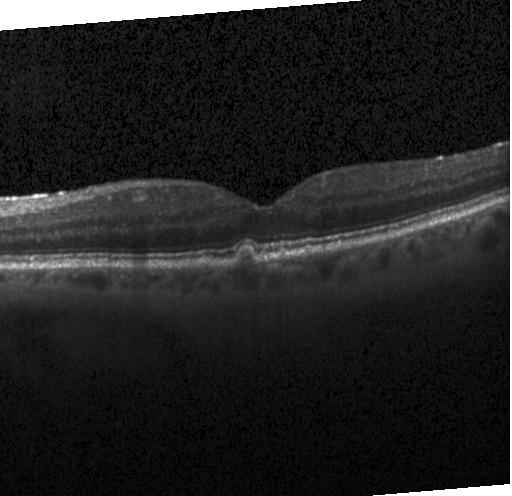 Impression: multiple drusen.